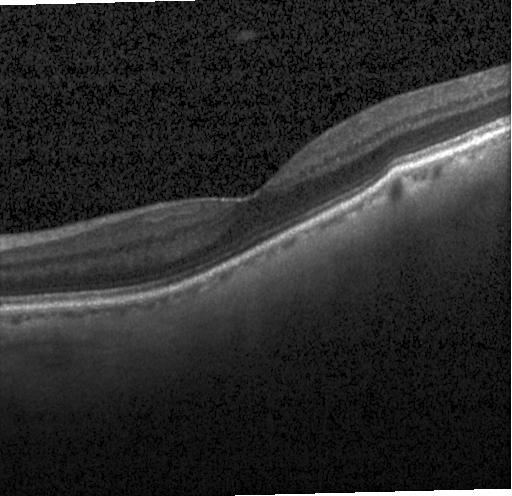
Retinal OCT cross-section showing no choroidal neovascularization, diabetic macular edema, or drusen.